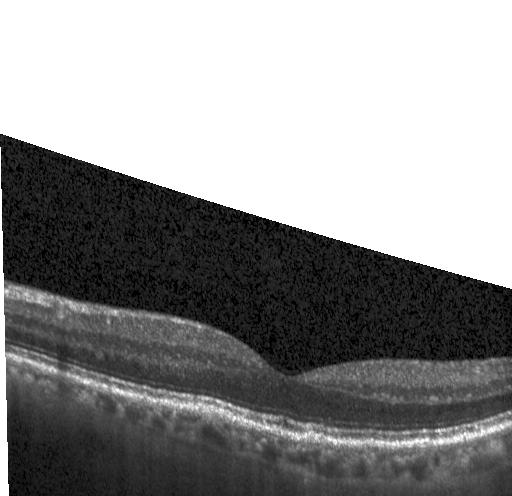 Acquired on a Heidelberg Spectralis · OCT line scan. Finding: no choroidal neovascularization, no diabetic macular edema, and no drusen.